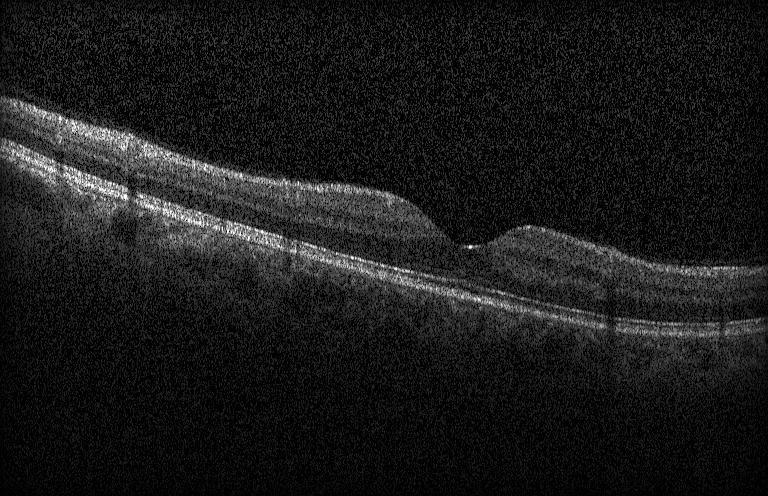 Acquired on a Heidelberg Spectralis; retinal OCT cross-section; spectral-domain optical coherence tomography.
Finding: no choroidal neovascularization, no diabetic macular edema, and no drusen.